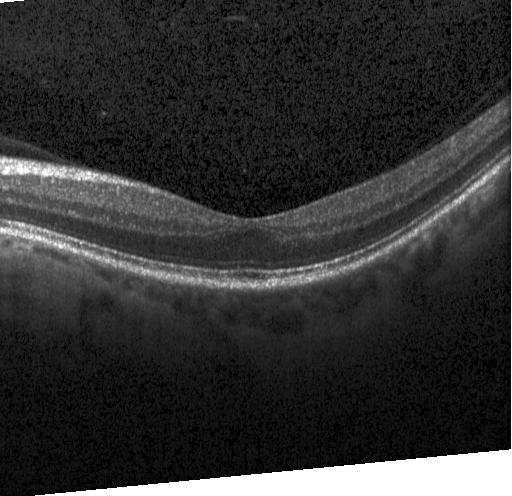
Retinal OCT B-scan; spectral-domain OCT; macular scan
OCT finding: no evidence of CNV, DME, or drusen.